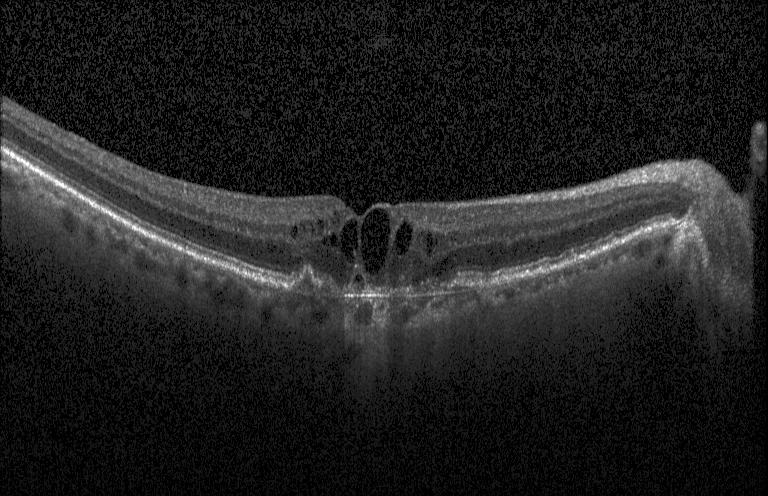 SD-OCT. Retinal OCT cross-section. Horizontal scan through the fovea — Diagnosis: choroidal neovascularization (CNV).